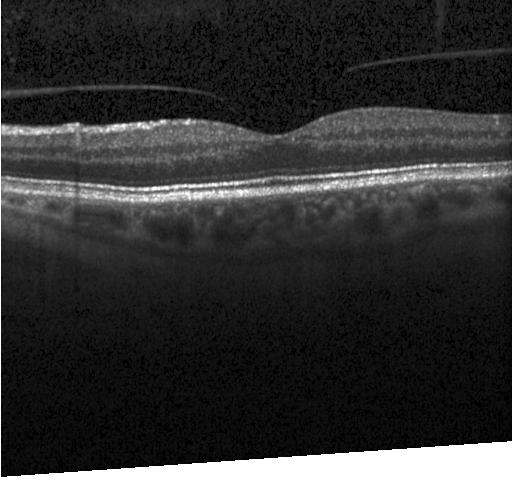
Macular OCT: neither choroidal neovascularization, diabetic macular edema, nor drusen.